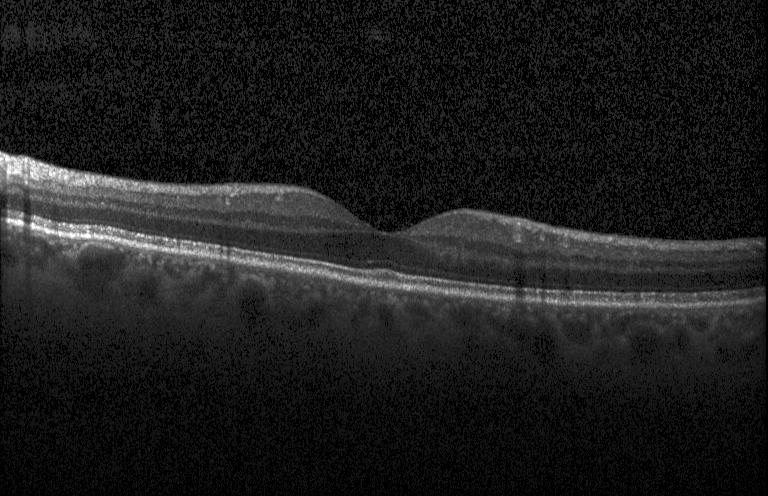 OCT B-scan, spectral-domain OCT, through the macula, Heidelberg Spectralis OCT system
Dx: no choroidal neovascularization, no diabetic macular edema, and no drusen.